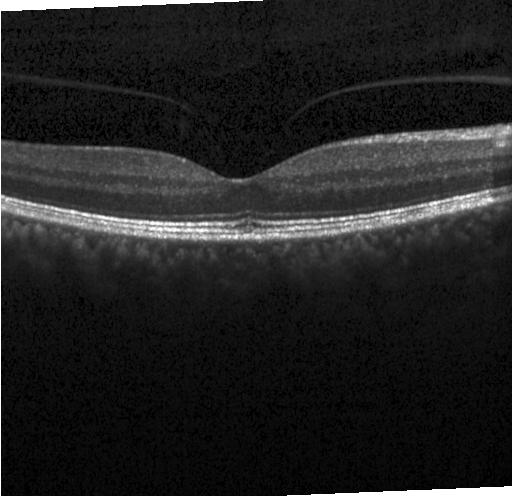
Retinal OCT cross-section — Diagnosis: no choroidal neovascularization, diabetic macular edema, or drusen.